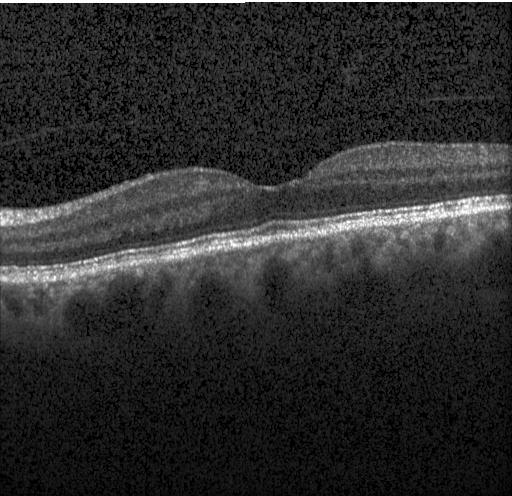
Macular OCT: neither choroidal neovascularization, diabetic macular edema, nor drusen.